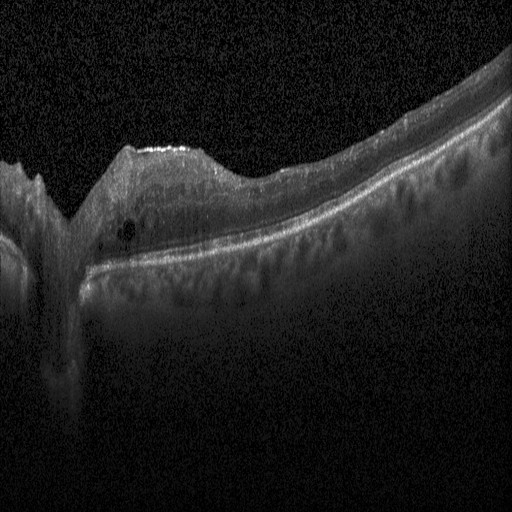
Spectral-domain OCT; optical coherence tomography scan.
Diabetic macular edema (DME).